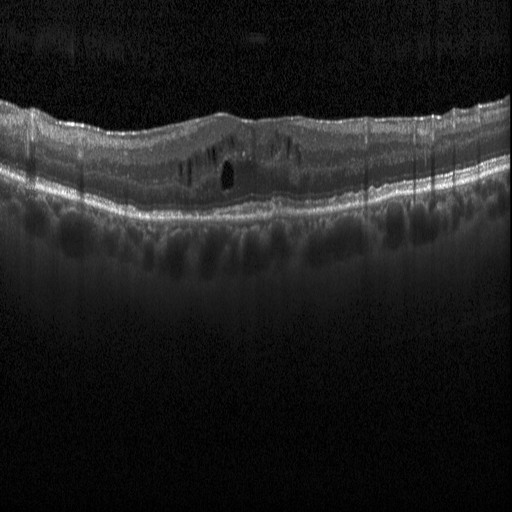

Spectral-domain optical coherence tomography, OCT line scan, horizontal scan through the fovea, instrument: Heidelberg Spectralis.
Diagnosis: diabetic macular edema.